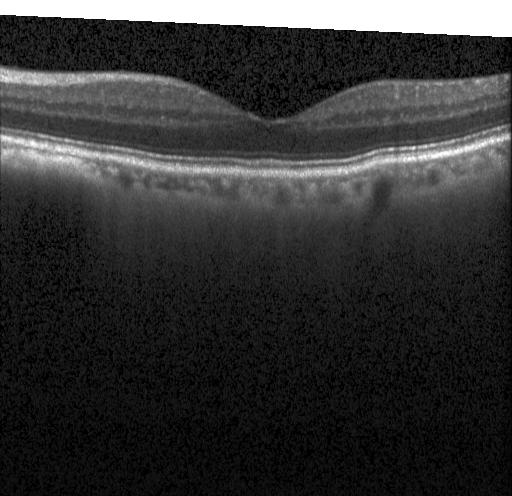 Optical coherence tomography scan. Finding: no evidence of choroidal neovascularization, diabetic macular edema, or drusen.